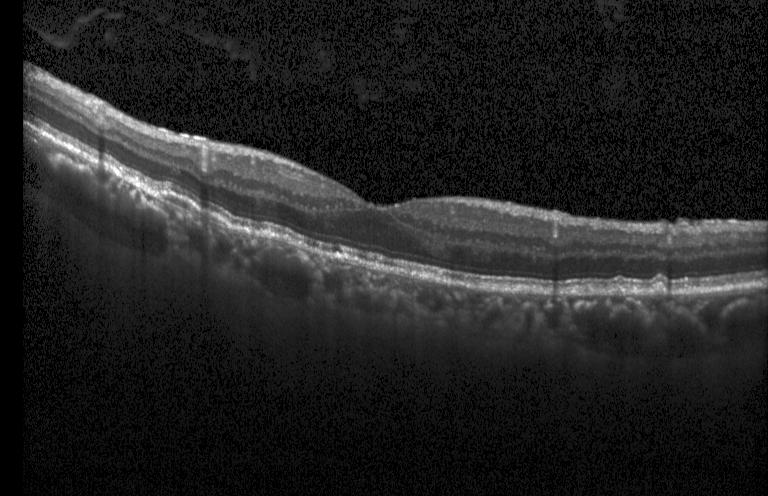
Finding: multiple drusen.